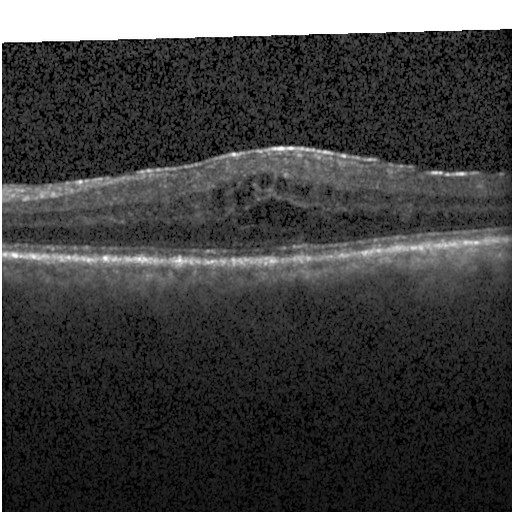

Finding: DME.